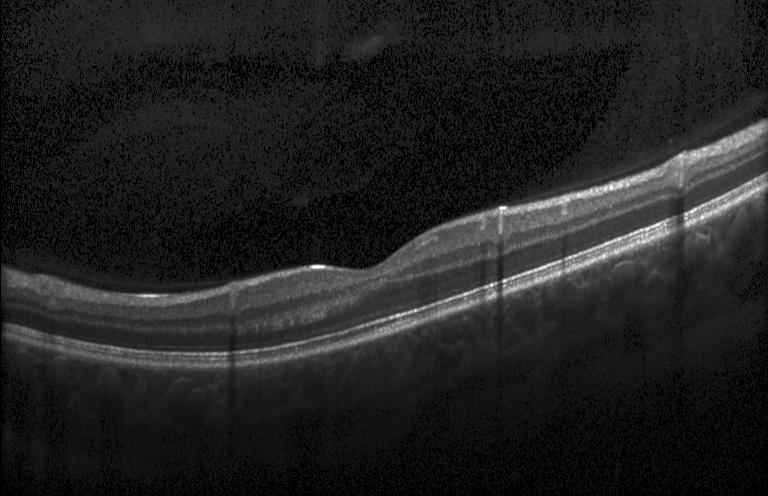 Retinal OCT cross-section showing no choroidal neovascularization, diabetic macular edema, or drusen.